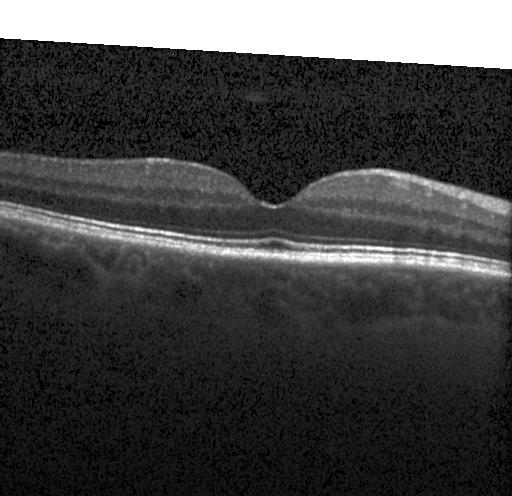 Optical coherence tomography B-scan.
Impression: neither choroidal neovascularization, diabetic macular edema, nor drusen.